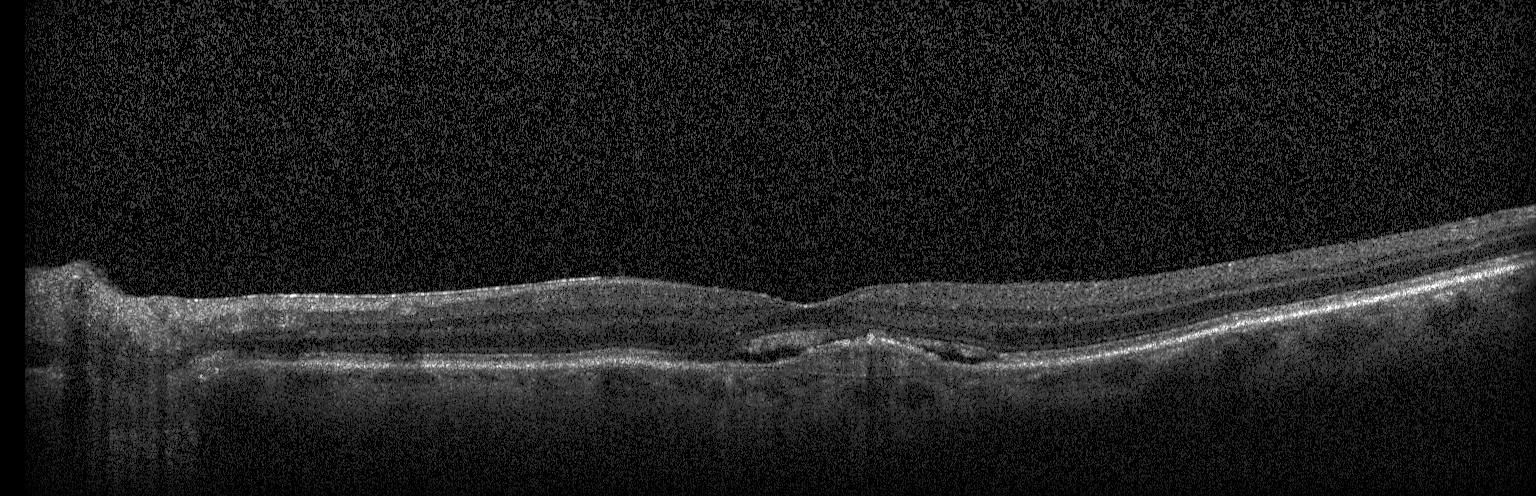

Retinal OCT B-scan
Diagnosis: choroidal neovascularization.